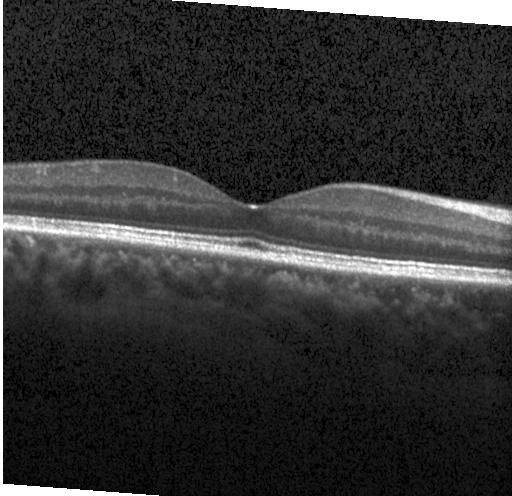
OCT B-scan showing no evidence of CNV, DME, or drusen.